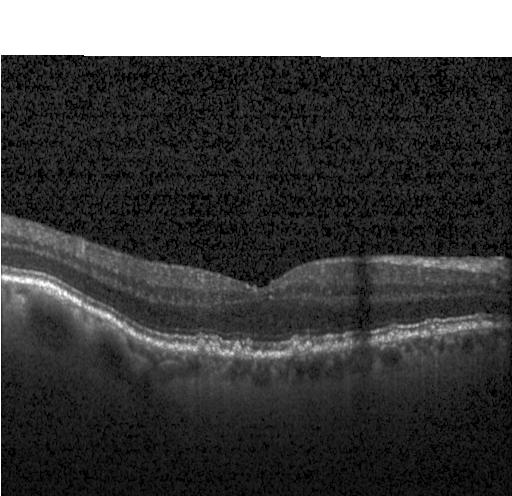

Instrument: Heidelberg Spectralis · retinal OCT B-scan · fovea-centered. Multiple drusen.